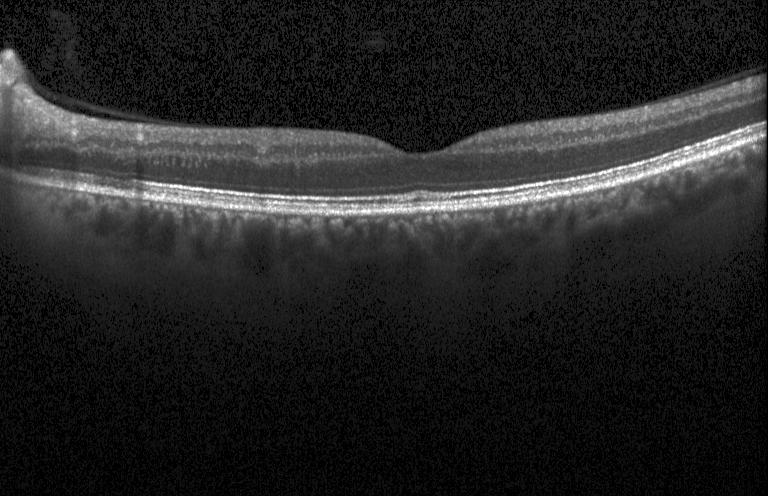

OCT scan showing no evidence of choroidal neovascularization, diabetic macular edema, or drusen.